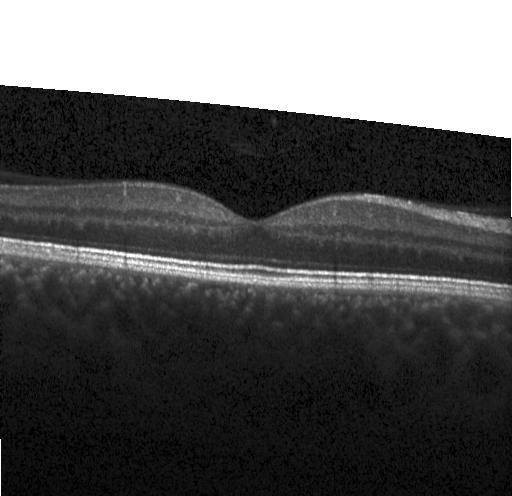 This B-scan demonstrates no choroidal neovascularization, no diabetic macular edema, and no drusen.